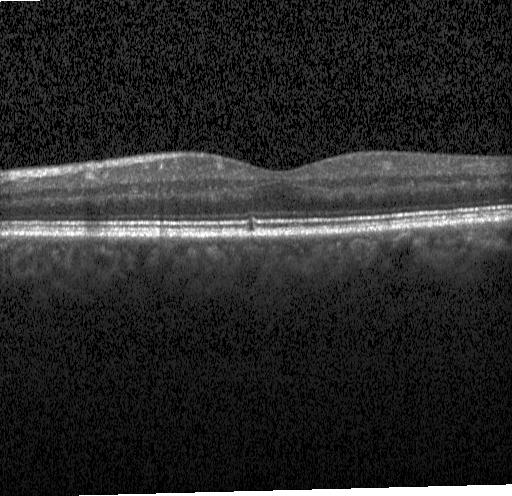 The scan shows no choroidal neovascularization, diabetic macular edema, or drusen.